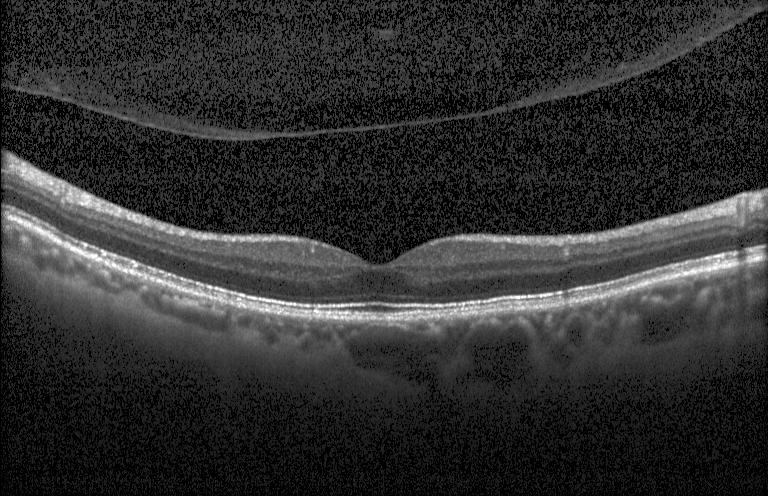 This B-scan demonstrates no choroidal neovascularization, diabetic macular edema, or drusen.